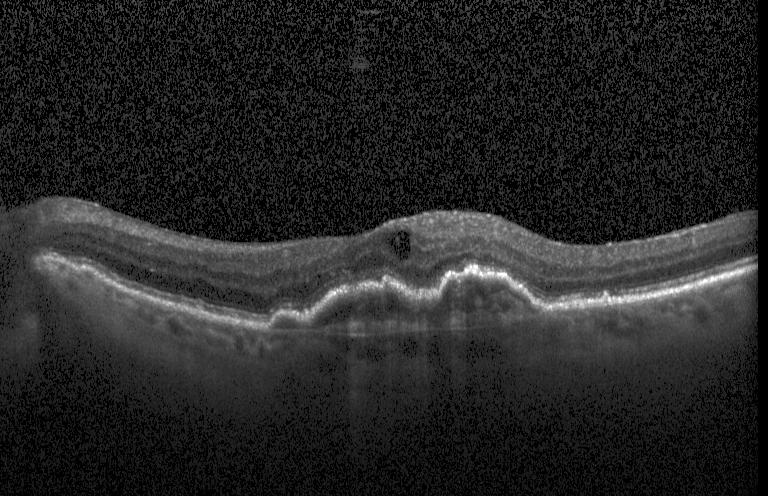
Impression: a choroidal neovascular membrane.